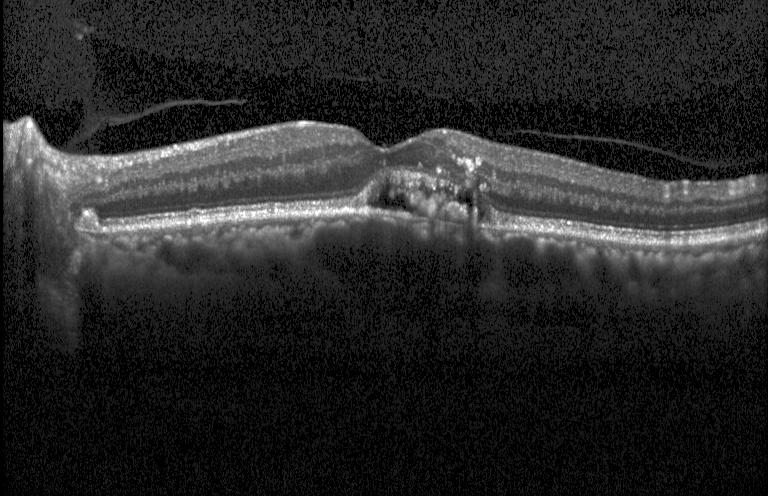
SD-OCT; OCT B-scan. The scan shows a choroidal neovascular membrane.